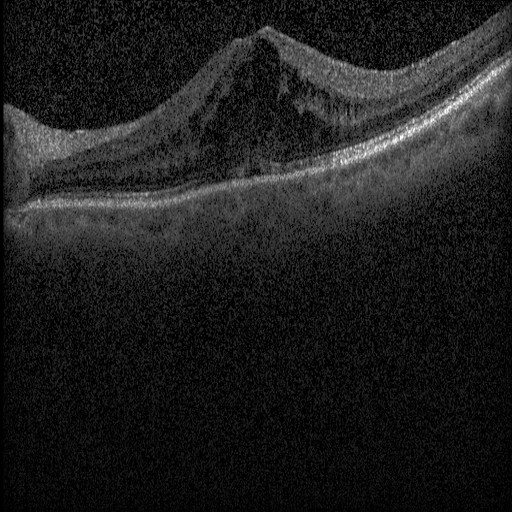
Retinal OCT B-scan · SD-OCT · macular scan.
Diagnosis: DME.